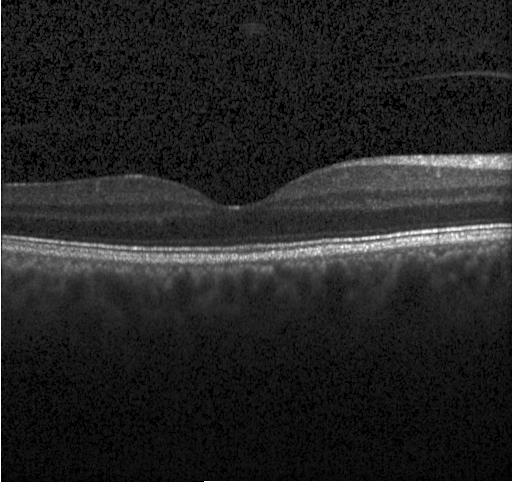

Heidelberg Spectralis OCT system. OCT line scan
This B-scan demonstrates no evidence of CNV, DME, or drusen.